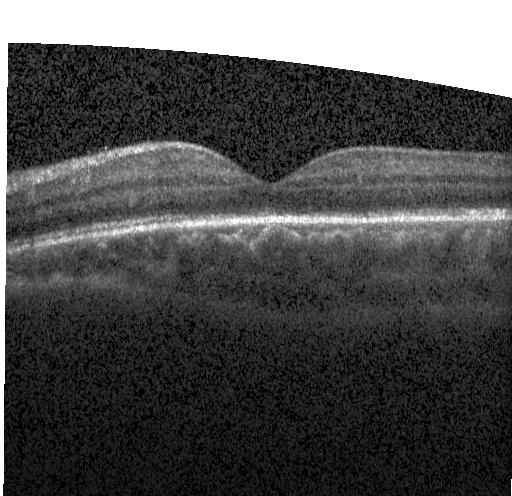

OCT scan showing no evidence of choroidal neovascularization, diabetic macular edema, or drusen.